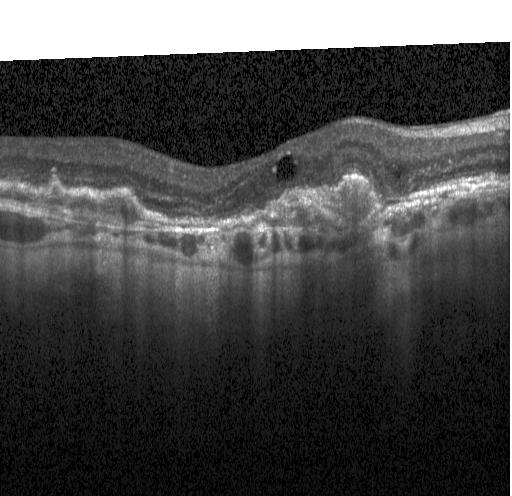 Heidelberg Spectralis OCT system; SD-OCT; horizontal scan through the fovea; OCT B-scan
Assessment: a choroidal neovascular membrane.